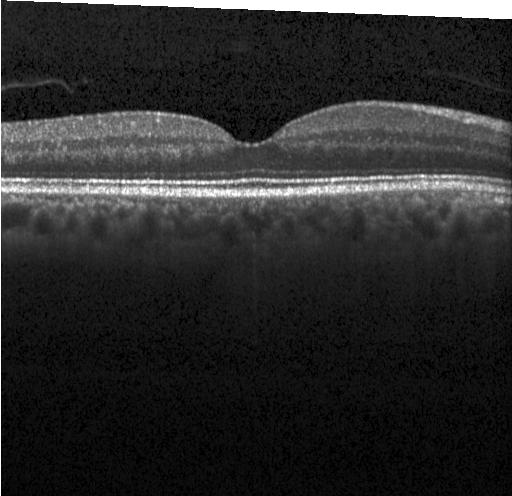
Dx: neither CNV, DME, nor drusen.